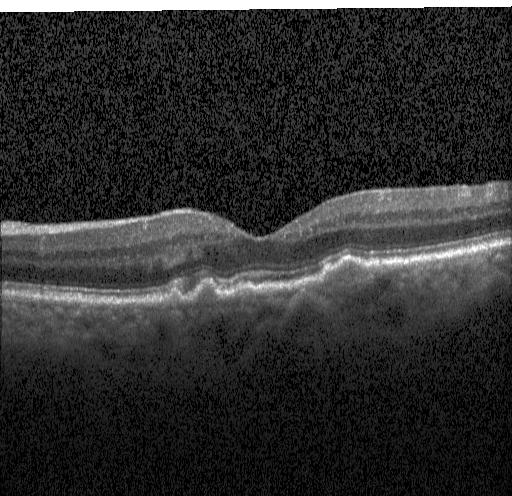

Optical coherence tomography scan. SD-OCT. Centered on the fovea — Finding: drusen.